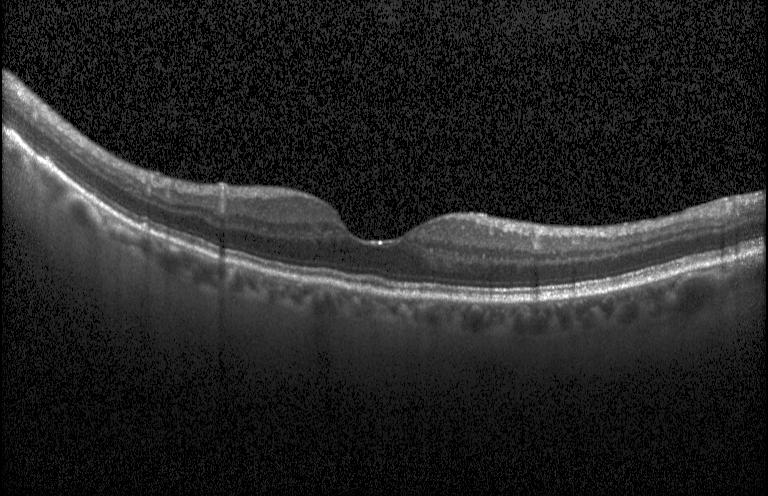
This B-scan demonstrates no choroidal neovascularization, no diabetic macular edema, and no drusen.